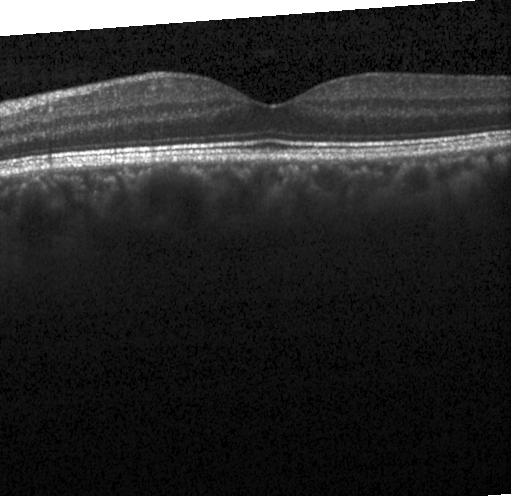 Retinal OCT B-scan; spectral-domain OCT; instrument: Heidelberg Spectralis.
This B-scan demonstrates no evidence of choroidal neovascularization, diabetic macular edema, or drusen.